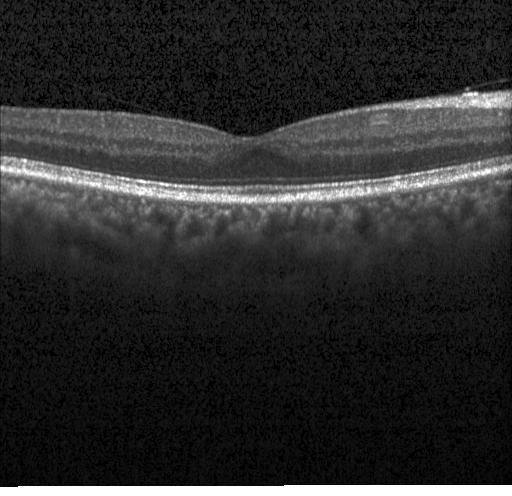

Macular OCT demonstrating no CNV, DME, or drusen.